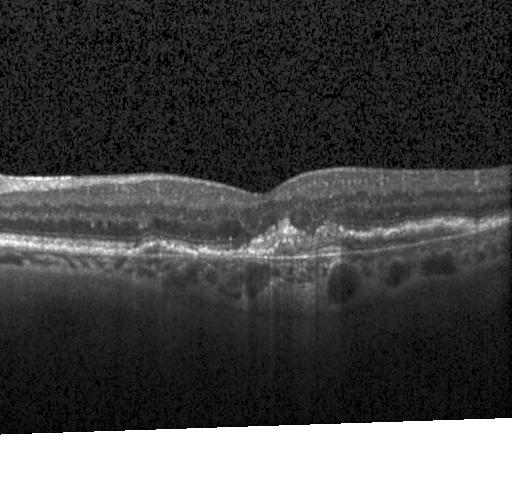
Assessment: choroidal neovascularization (CNV).